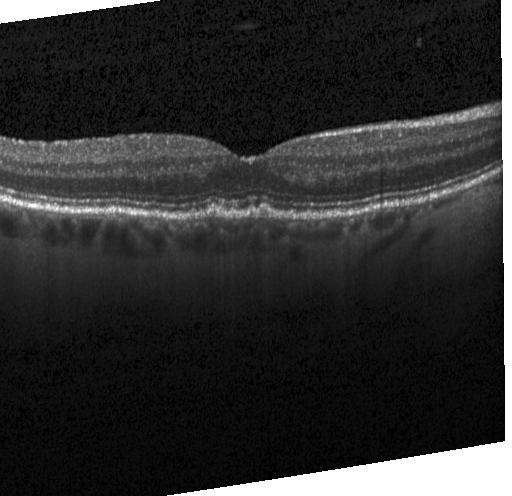

Diagnosis: sub-RPE drusenoid deposits.